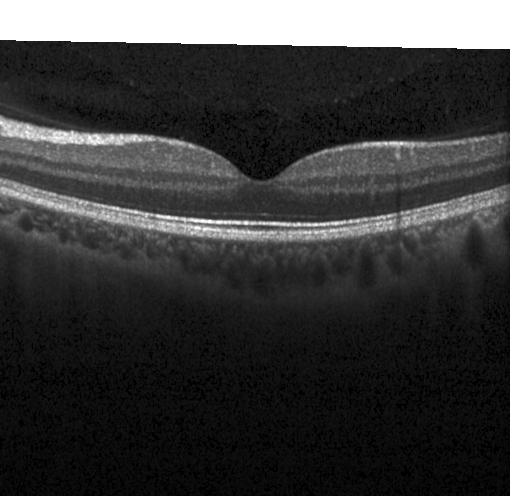
Optical coherence tomography B-scan — Diagnosis: no choroidal neovascularization, no diabetic macular edema, and no drusen.